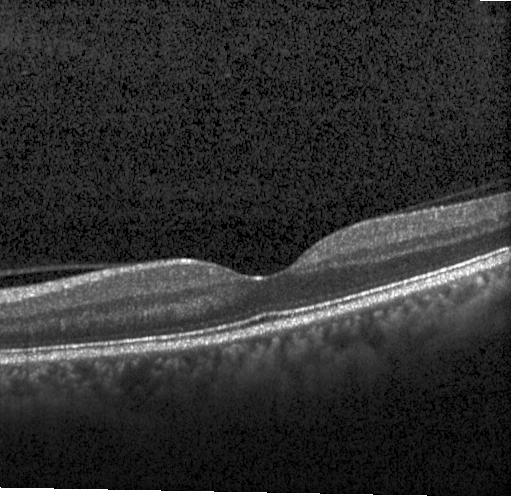 Horizontal scan through the fovea. Spectral-domain optical coherence tomography. Optical coherence tomography scan. Heidelberg Spectralis OCT system. Assessment: no CNV, DME, or drusen.